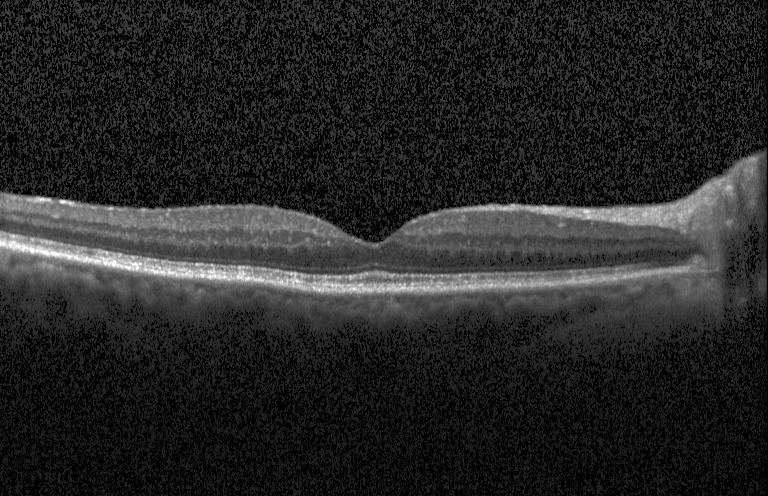

SD-OCT, retinal OCT cross-section, centered on the fovea.
Diagnosis: no choroidal neovascularization, no diabetic macular edema, and no drusen.